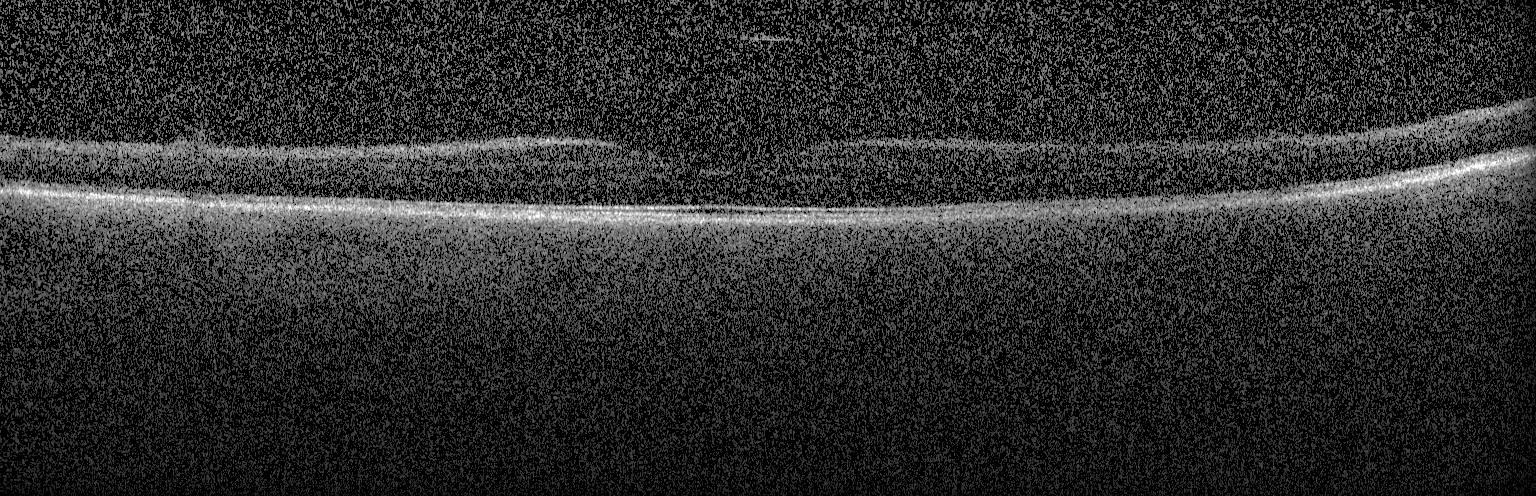

Retinal OCT cross-section
Impression: no CNV, DME, or drusen.